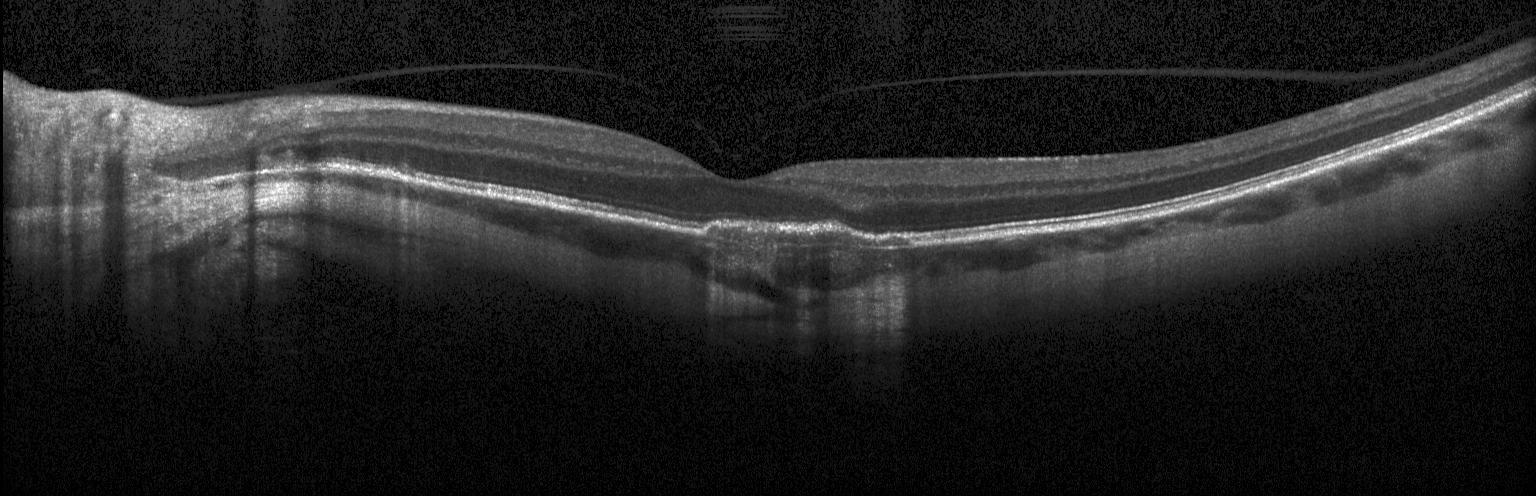 Optical coherence tomography scan; Heidelberg Spectralis OCT system. Finding: choroidal neovascularization (CNV).